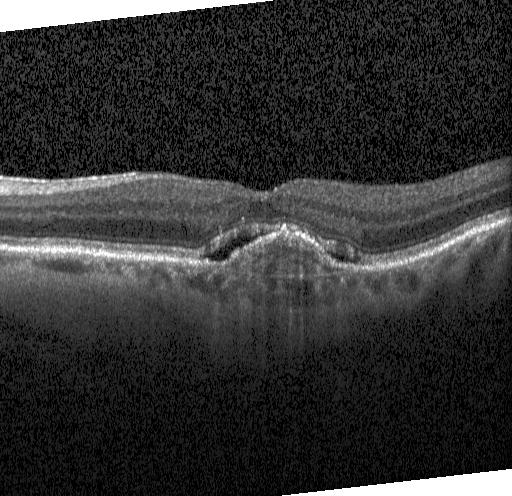
Optical coherence tomography B-scan. Instrument: Heidelberg Spectralis.
Diagnosis: a choroidal neovascular membrane.